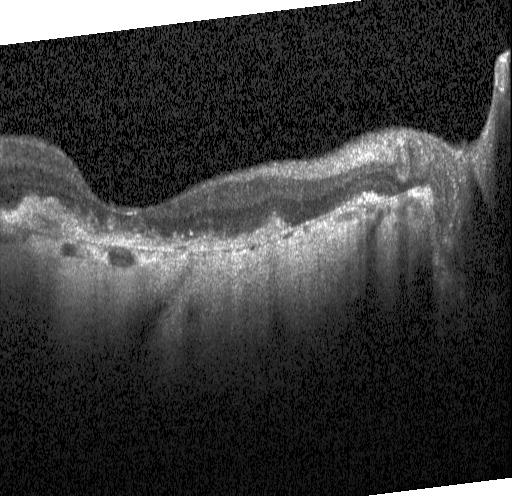 Spectral-domain OCT B-scan: a choroidal neovascular membrane.